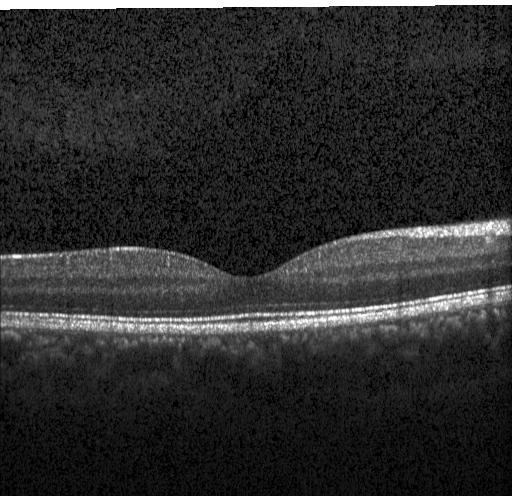

Optical coherence tomography B-scan. Spectral-domain optical coherence tomography. Horizontal scan through the fovea. Acquired on a Heidelberg Spectralis.
Impression: no choroidal neovascularization, diabetic macular edema, or drusen.